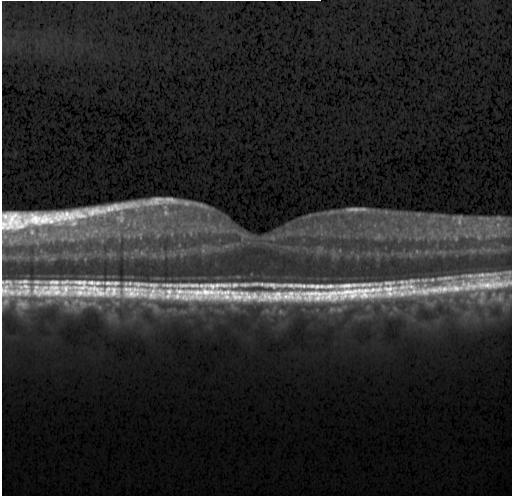 OCT line scan — OCT finding: neither choroidal neovascularization, diabetic macular edema, nor drusen.